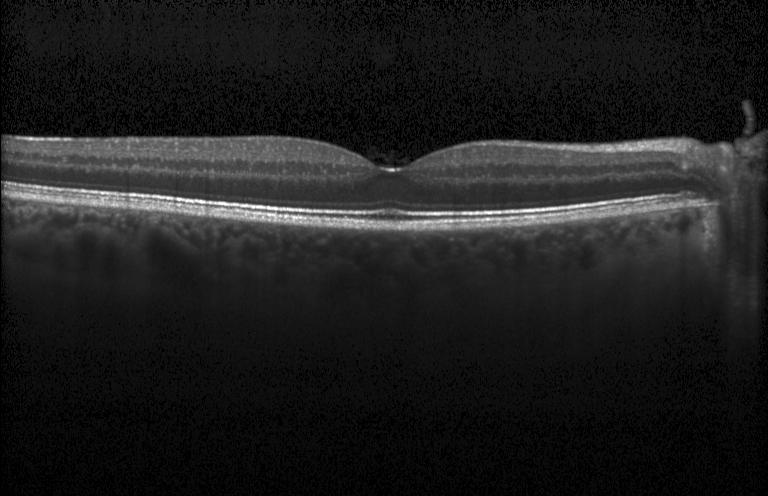

SD-OCT. Retinal OCT B-scan. Diagnosis: no choroidal neovascularization, no diabetic macular edema, and no drusen.